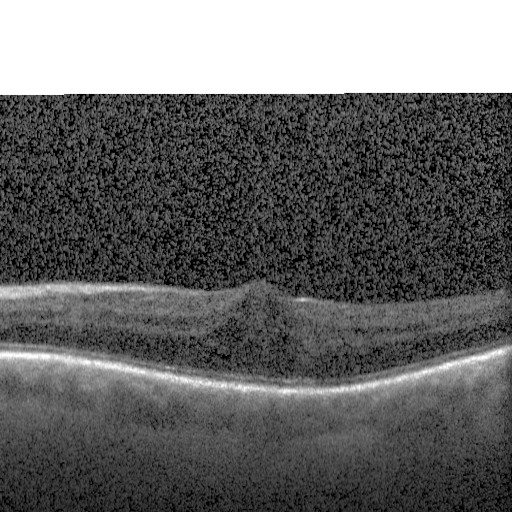

Macular OCT: DME.